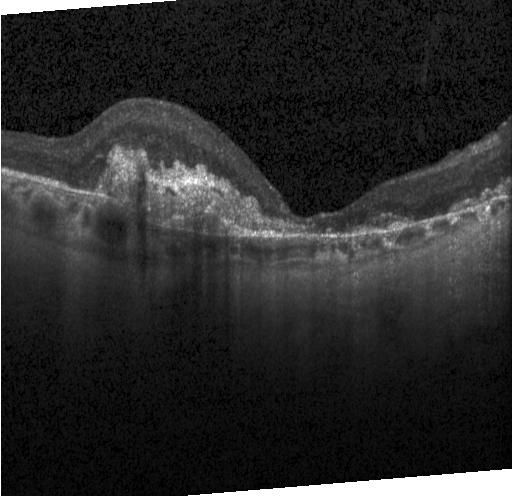

OCT B-scan showing a choroidal neovascular membrane.